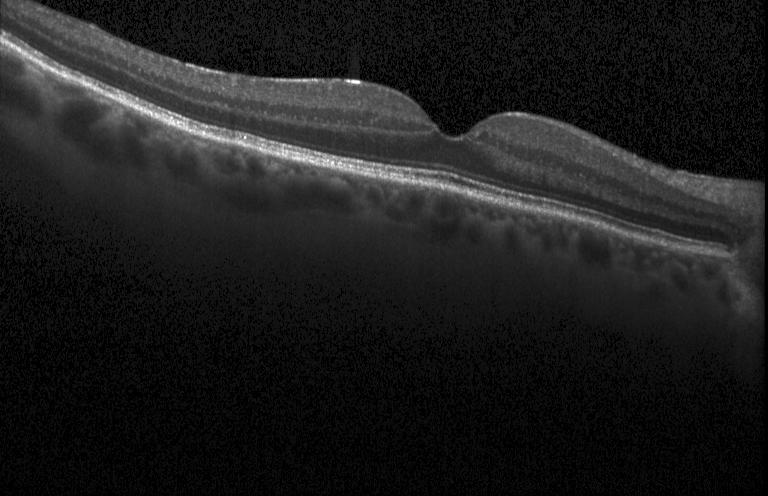

Heidelberg Spectralis OCT system; SD-OCT; optical coherence tomography scan. Impression: neither choroidal neovascularization, diabetic macular edema, nor drusen.